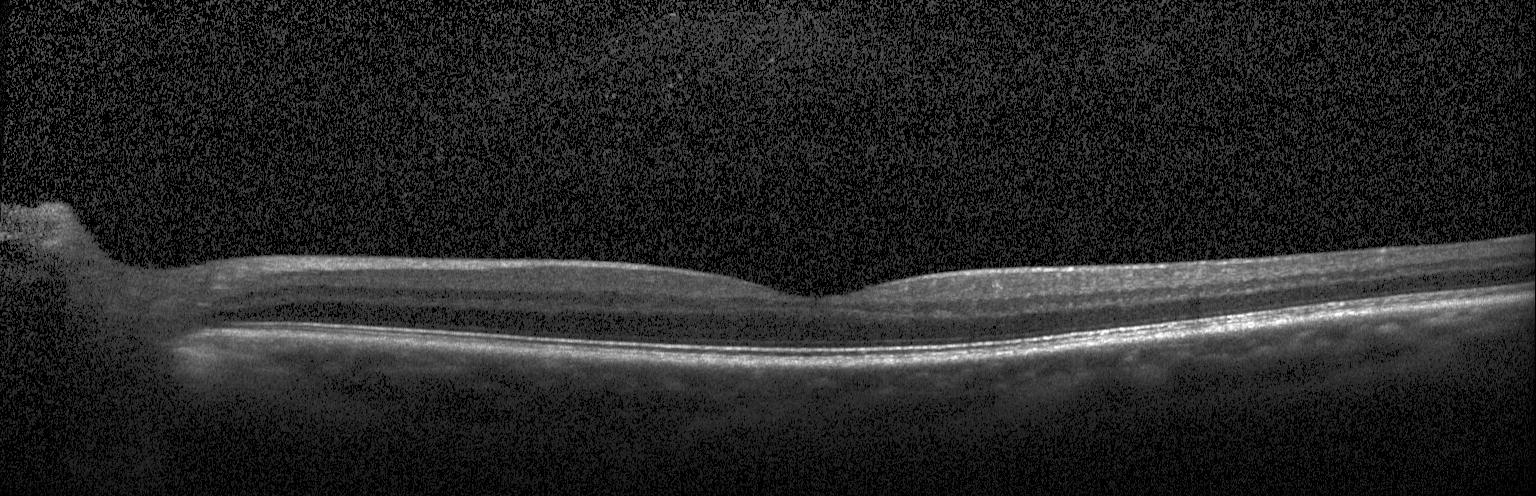
Optical coherence tomography scan
Impression: neither choroidal neovascularization, diabetic macular edema, nor drusen.